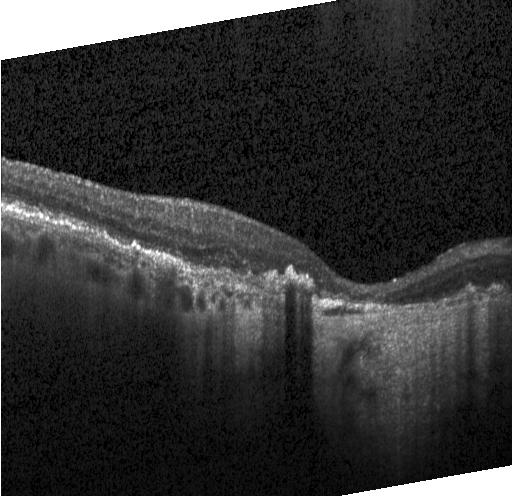 Retinal OCT cross-section, acquired on a Heidelberg Spectralis.
Impression: a choroidal neovascular membrane.